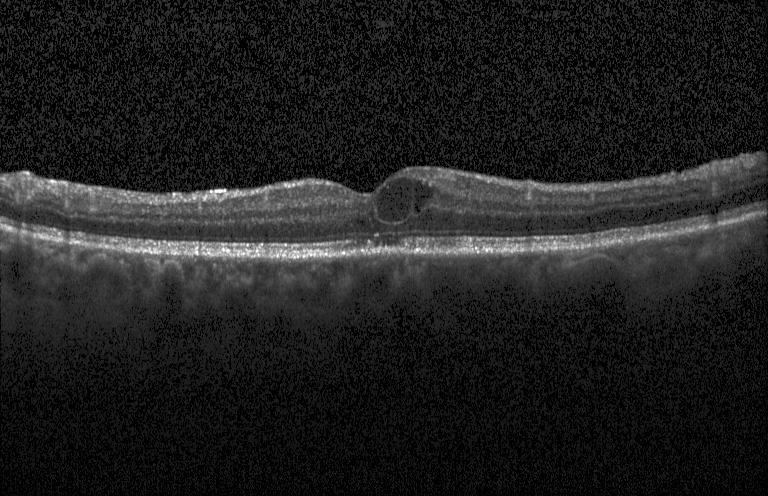
OCT B-scan · Heidelberg Spectralis · macular scan.
OCT finding: diabetic macular edema.